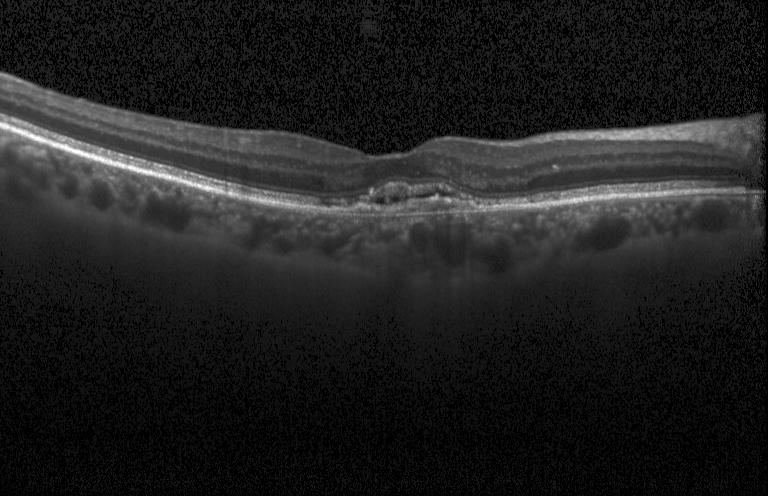

Diagnosis: a choroidal neovascular membrane.